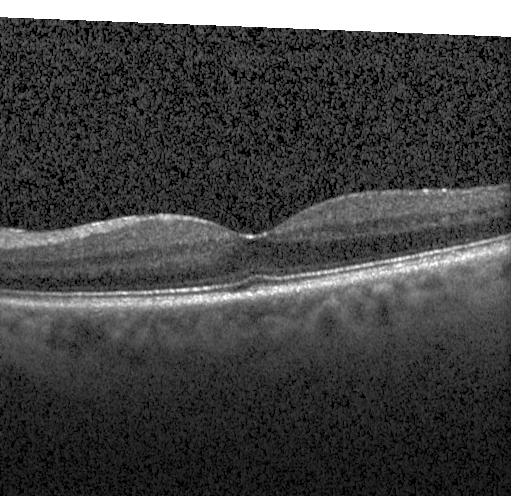
Macular OCT demonstrating no choroidal neovascularization, diabetic macular edema, or drusen.